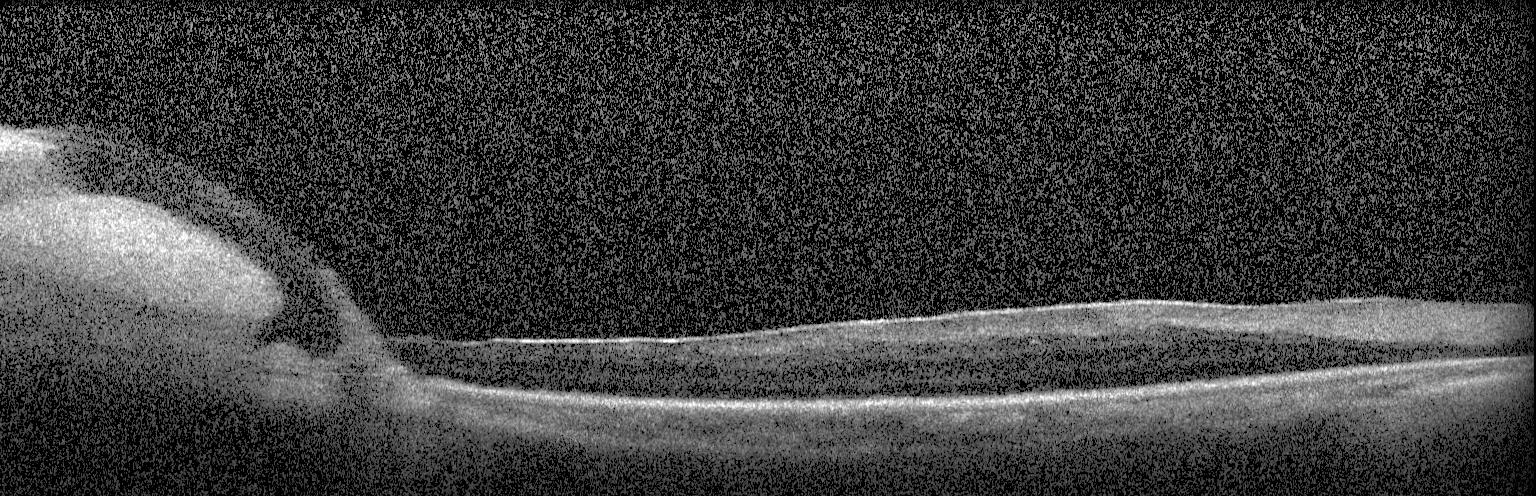

Macular OCT: a choroidal neovascular membrane.